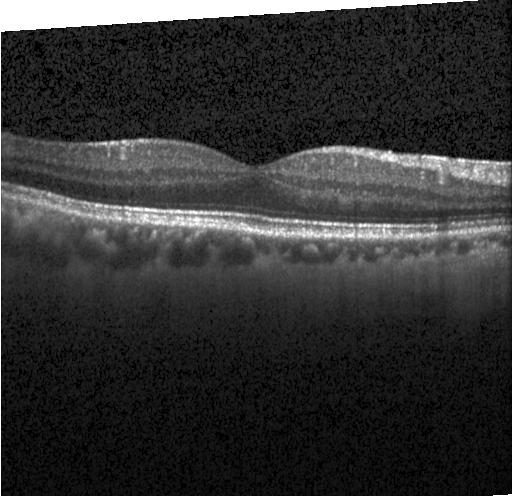

OCT line scan, acquired on a Heidelberg Spectralis. The scan shows no choroidal neovascularization, no diabetic macular edema, and no drusen.